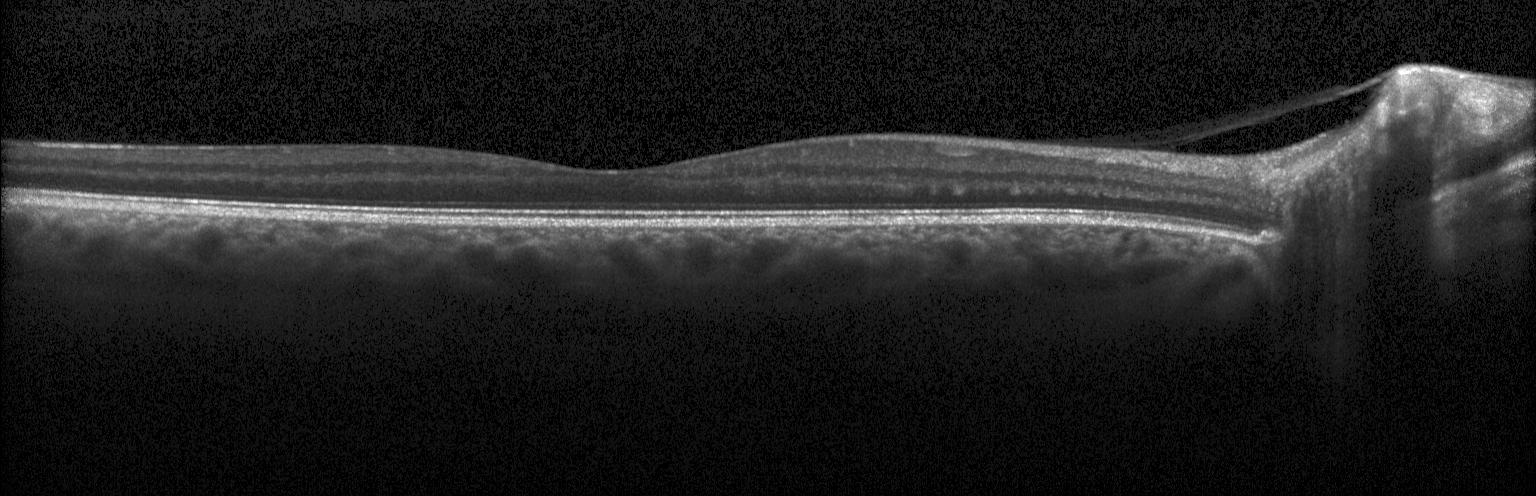
SD-OCT; retinal OCT B-scan; macular scan; Heidelberg Spectralis.
Dx: neither CNV, DME, nor drusen.